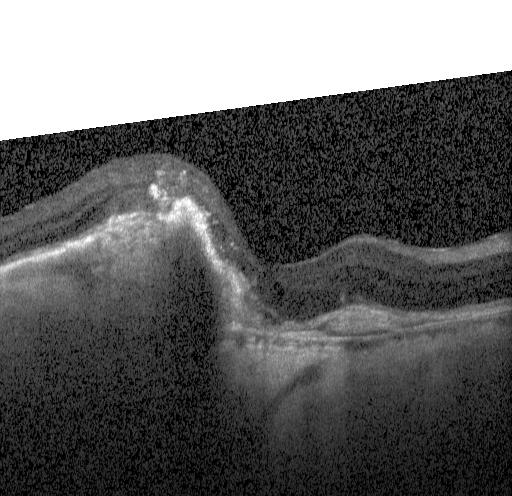 Optical coherence tomography scan. Spectral-domain OCT. Macular scan. Acquired on a Heidelberg Spectralis — Macular OCT: a choroidal neovascular membrane.